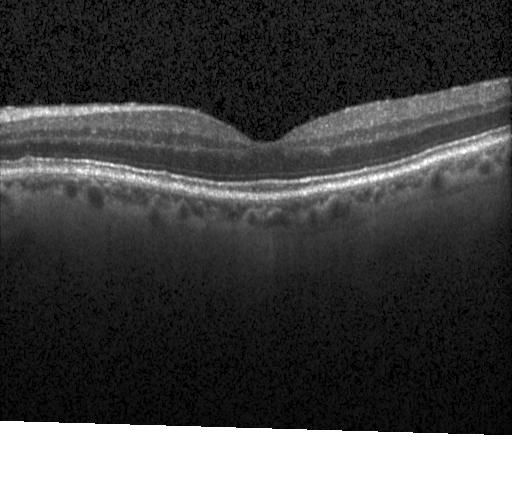
OCT line scan, spectral-domain optical coherence tomography, Heidelberg Spectralis, fovea-centered — Diagnosis: no CNV, DME, or drusen.